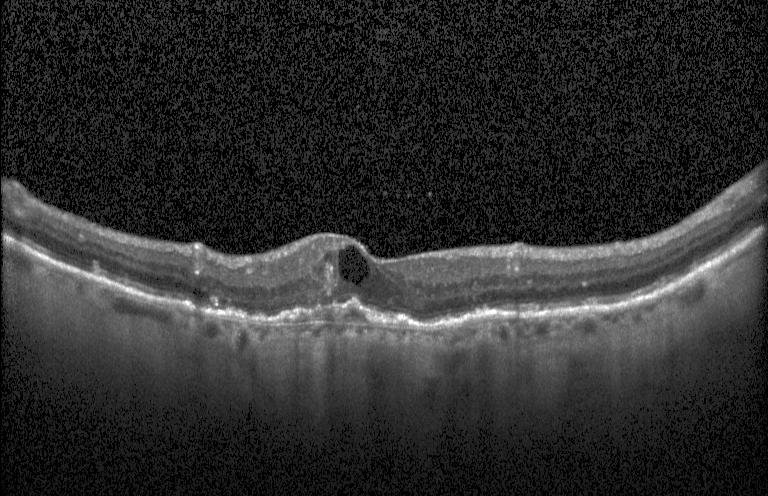

The scan shows a choroidal neovascular membrane.